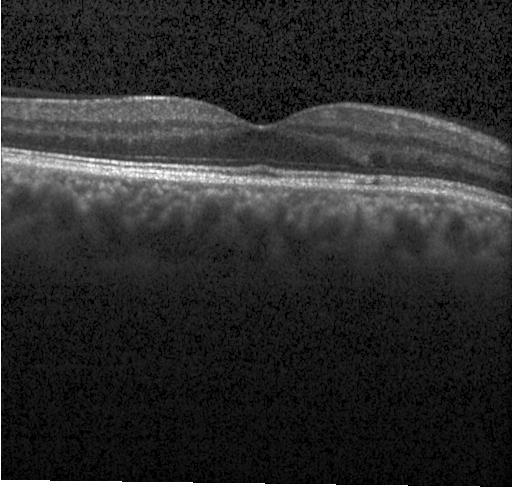

OCT line scan — OCT finding: no choroidal neovascularization, diabetic macular edema, or drusen.